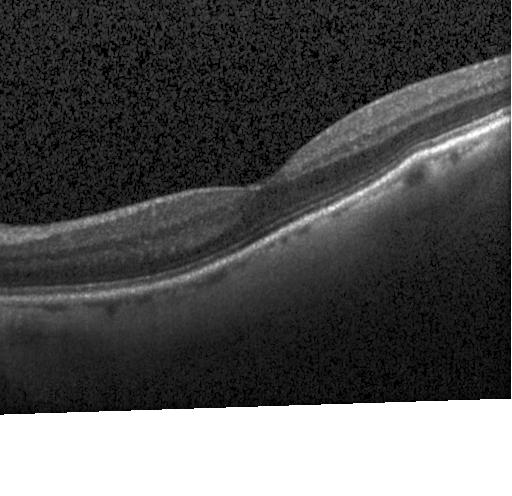 Impression: neither choroidal neovascularization, diabetic macular edema, nor drusen.